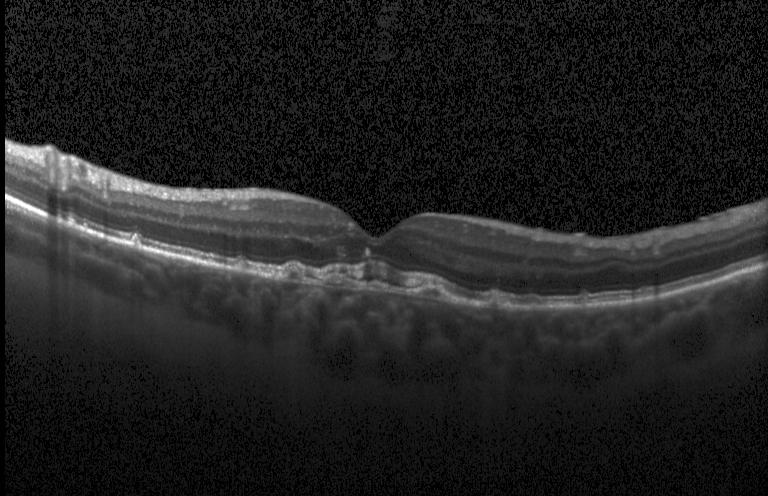
OCT scan showing CNV.